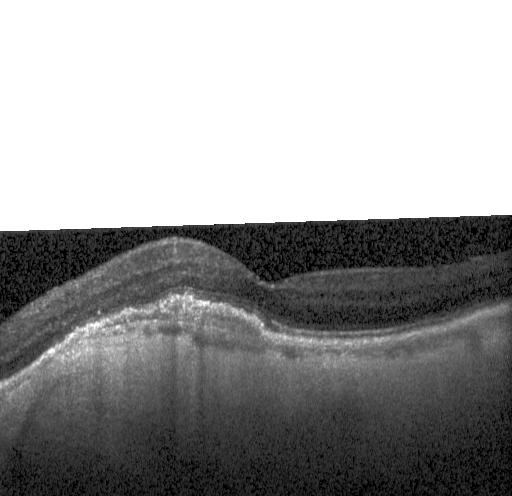 Macular OCT demonstrating a choroidal neovascular membrane.